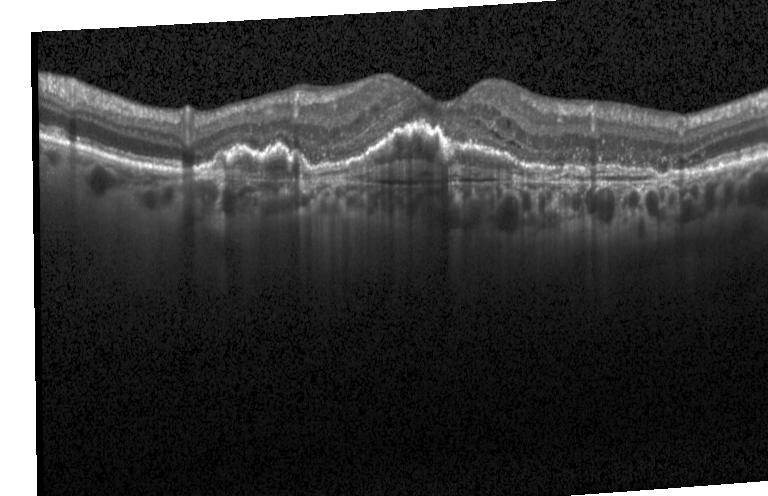 OCT B-scan — This B-scan demonstrates a choroidal neovascular membrane.